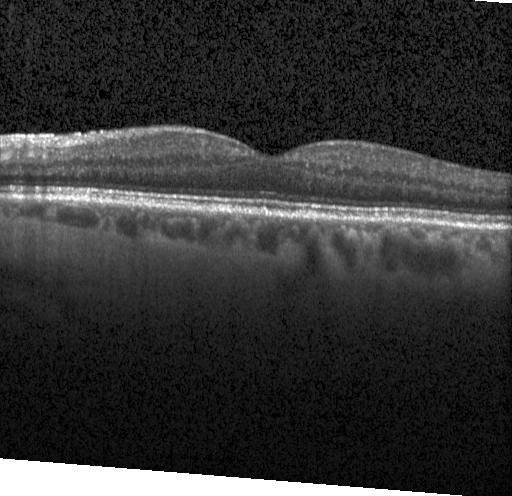

Retinal OCT cross-section.
Macular OCT: no CNV, DME, or drusen.